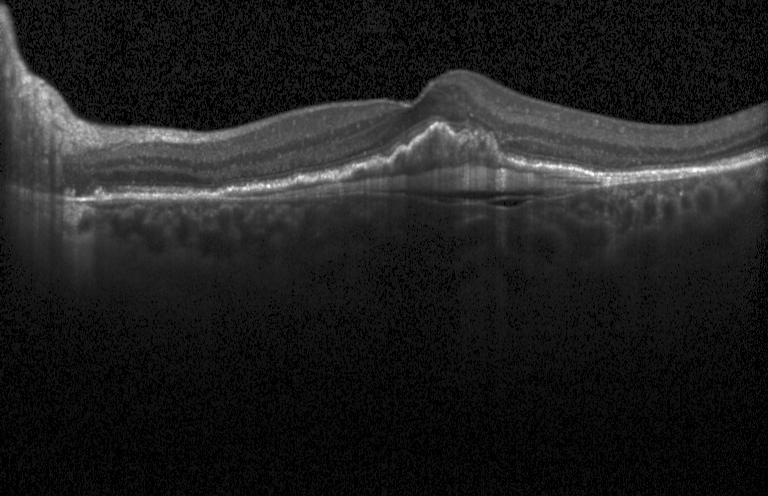 Dx: CNV.